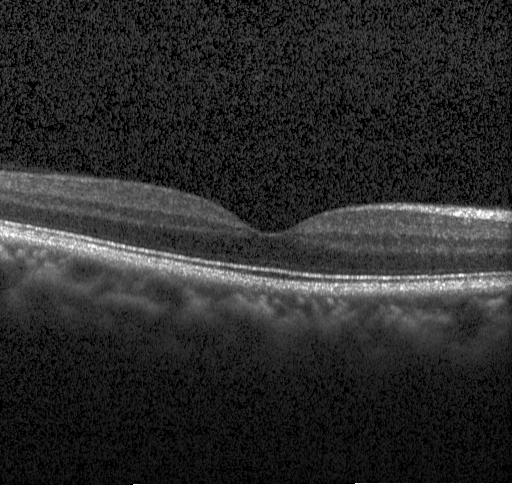 OCT B-scan.
Impression: no CNV, no DME, and no drusen.